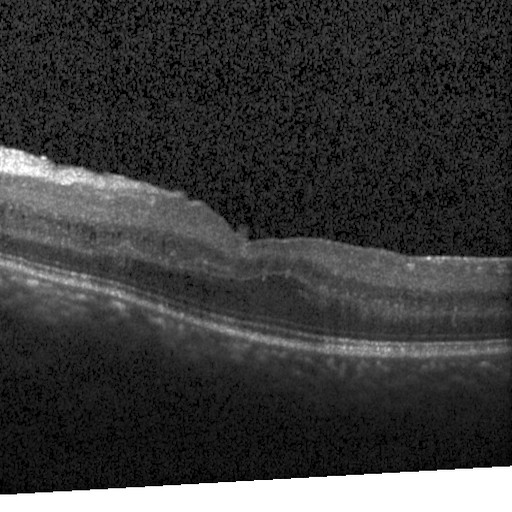
Finding: diabetic macular edema (DME).